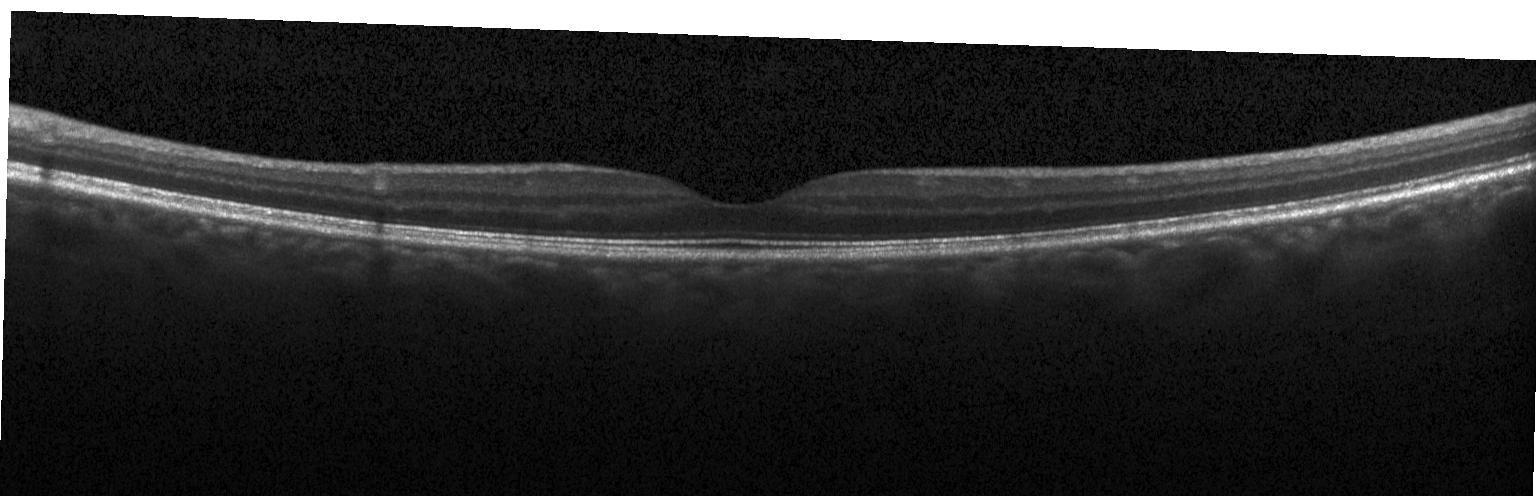

SD-OCT, OCT B-scan, macular scan.
This B-scan demonstrates neither choroidal neovascularization, diabetic macular edema, nor drusen.